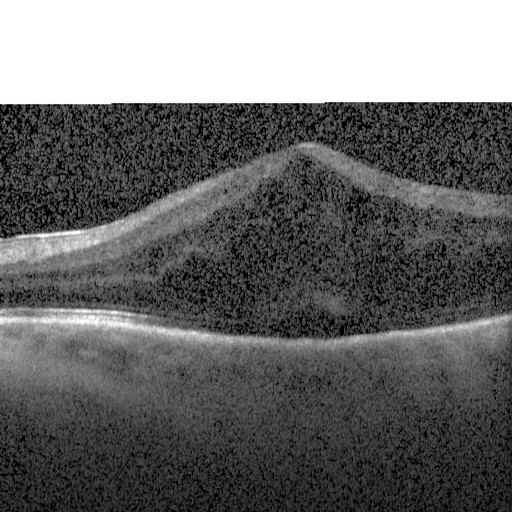

Optical coherence tomography B-scan. Assessment: diabetic macular edema.